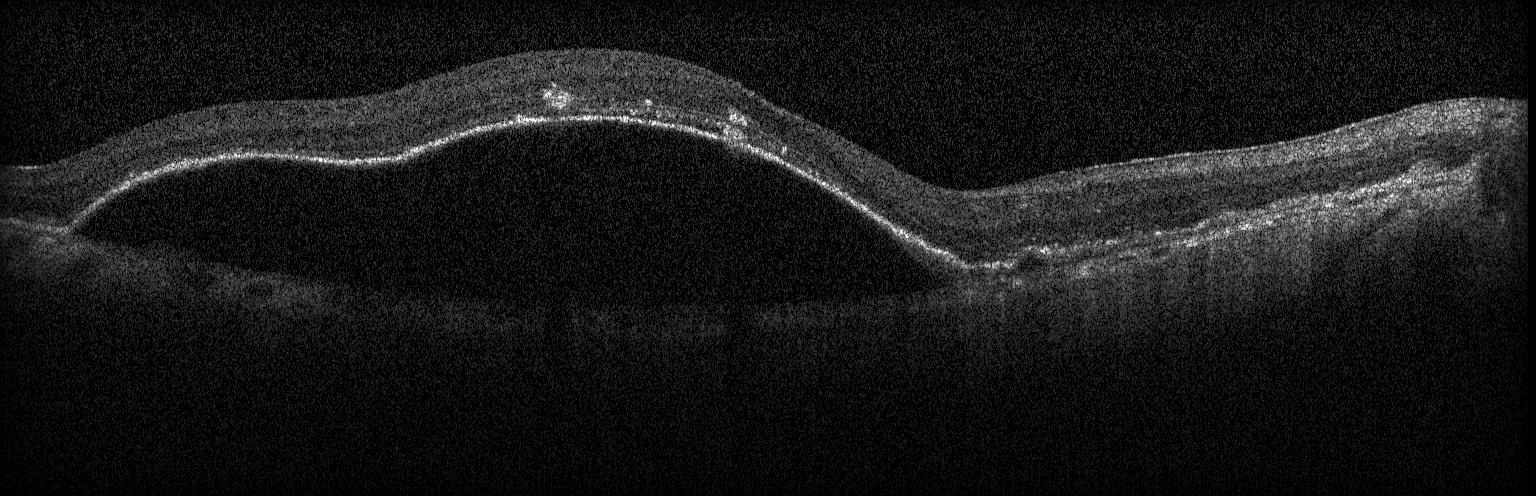
The scan shows choroidal neovascularization (CNV).